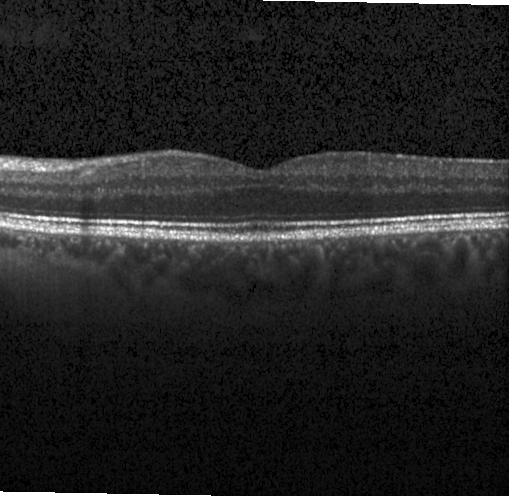
Horizontal scan through the fovea · Heidelberg Spectralis OCT system · SD-OCT · optical coherence tomography B-scan.
The scan shows no choroidal neovascularization, no diabetic macular edema, and no drusen.